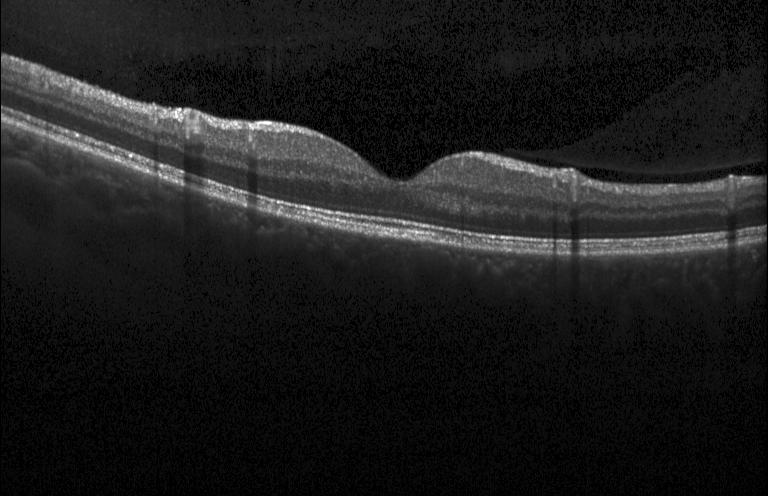

Optical coherence tomography scan. This B-scan demonstrates no evidence of choroidal neovascularization, diabetic macular edema, or drusen.